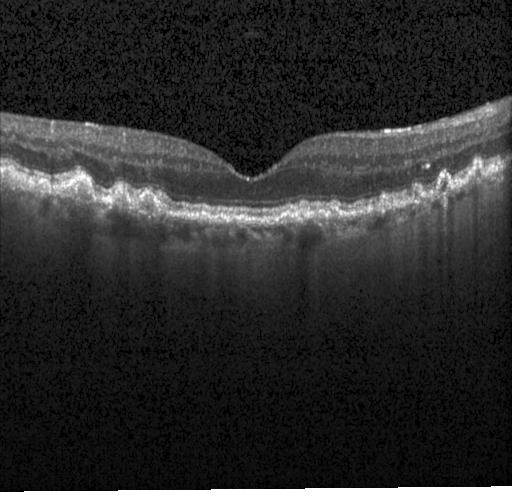 OCT B-scan · spectral-domain OCT · instrument: Heidelberg Spectralis · through the macula
Impression: sub-RPE drusenoid deposits.